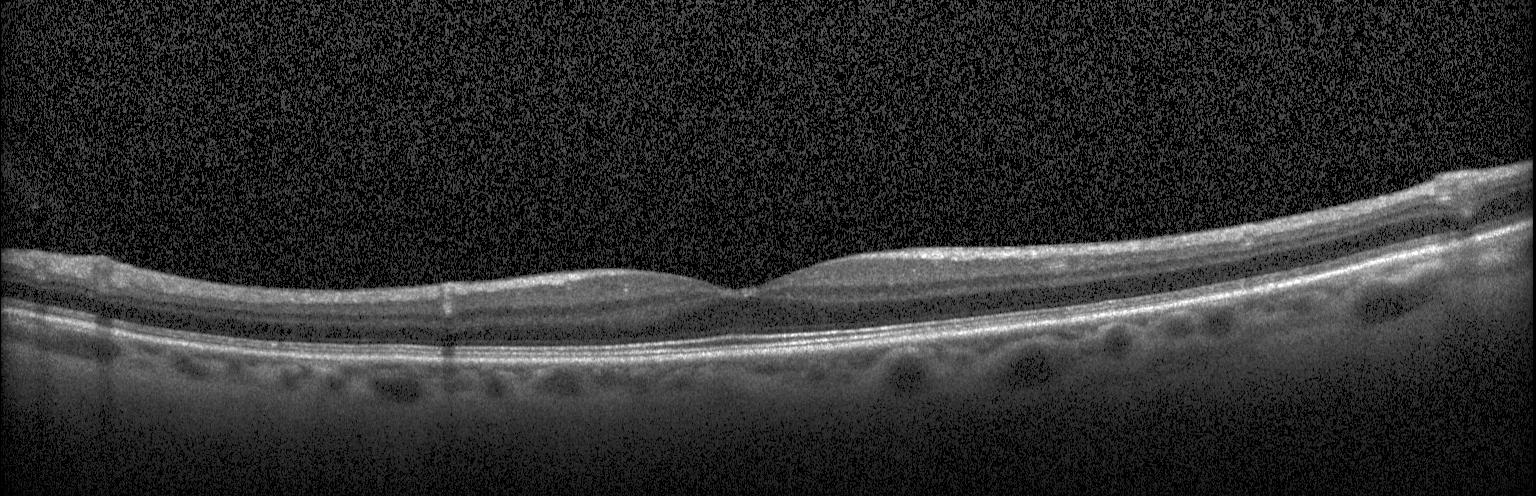

Finding: no evidence of CNV, DME, or drusen.